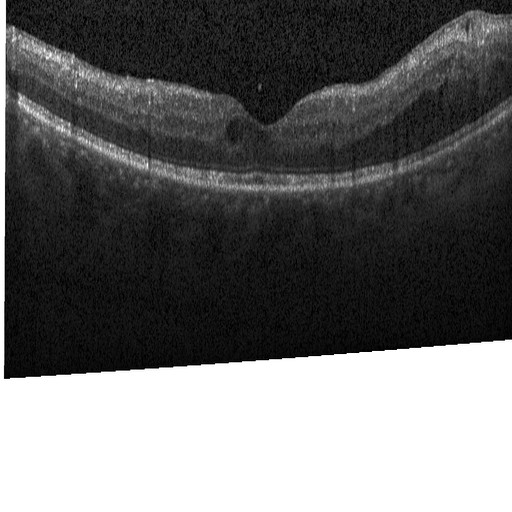
OCT finding: diabetic macular edema (DME).